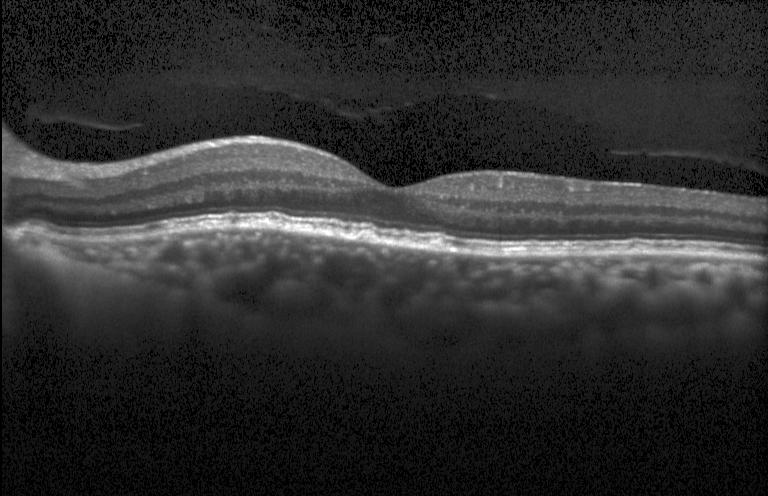

Macular OCT: sub-RPE drusenoid deposits.